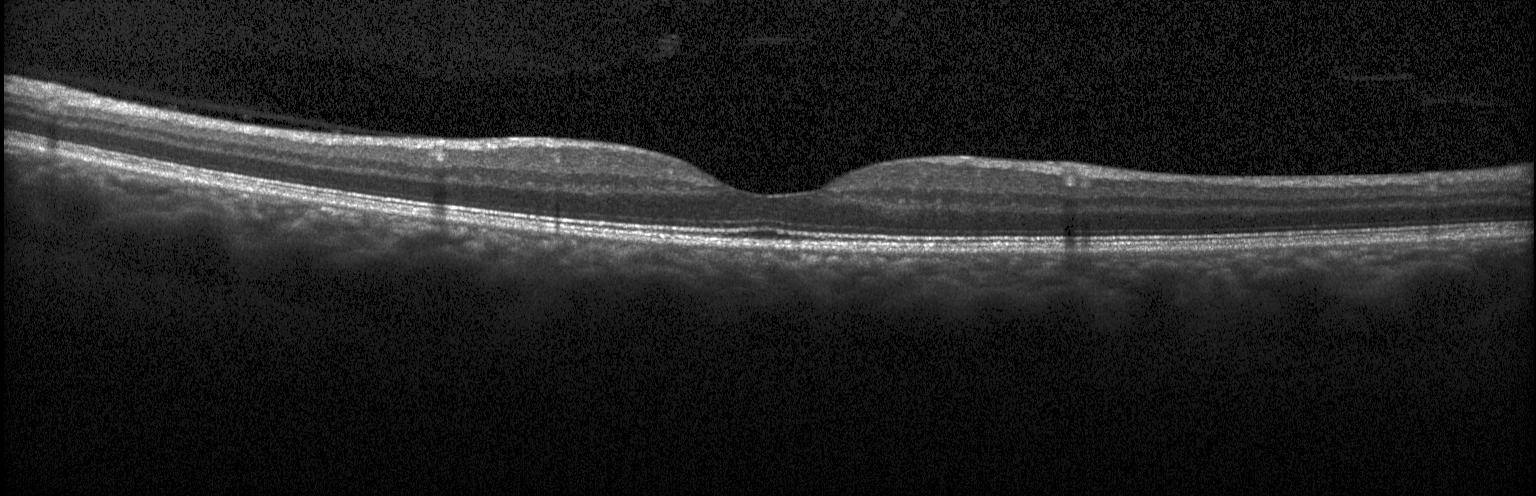
OCT B-scan showing neither CNV, DME, nor drusen.